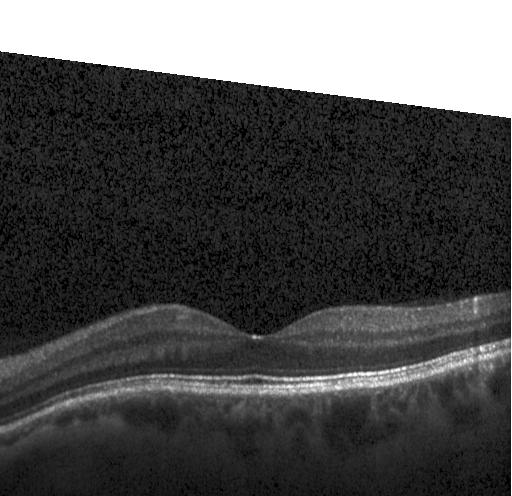

Diagnosis: no choroidal neovascularization, diabetic macular edema, or drusen.